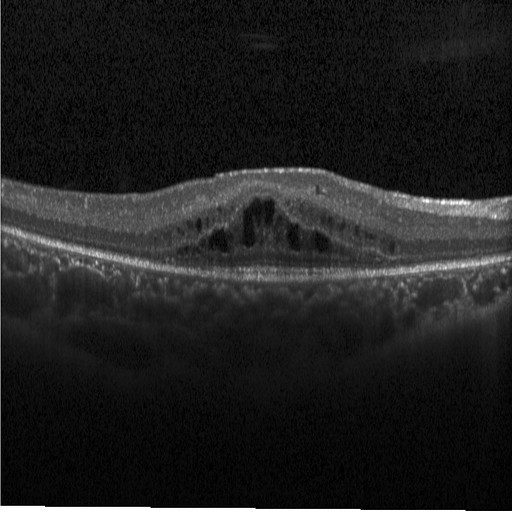 OCT line scan · Heidelberg Spectralis — OCT finding: diabetic macular edema (DME).